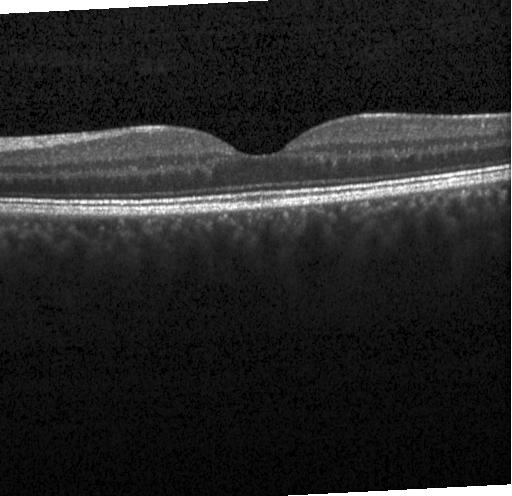
Diagnosis: no evidence of choroidal neovascularization, diabetic macular edema, or drusen.